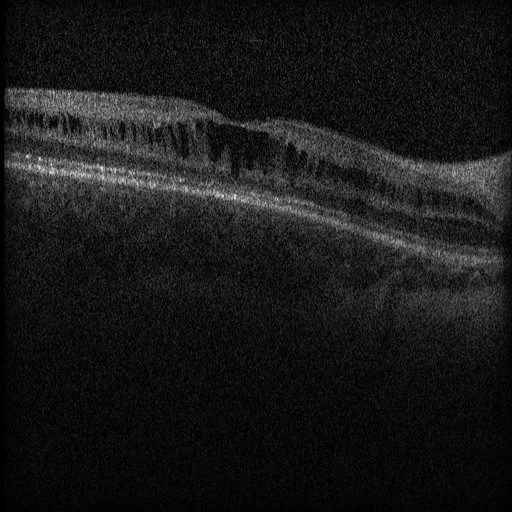

OCT finding: DME.